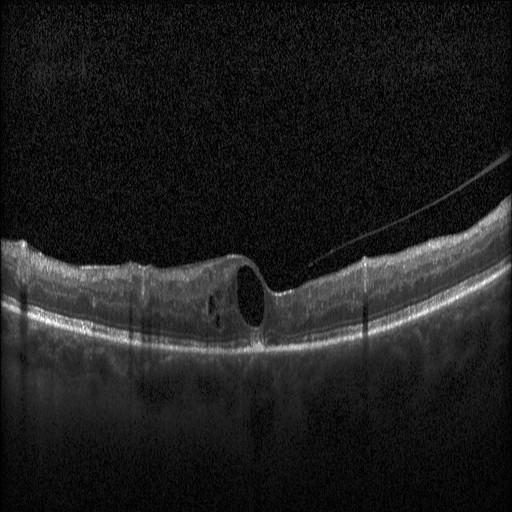
Impression: diabetic macular edema (DME).